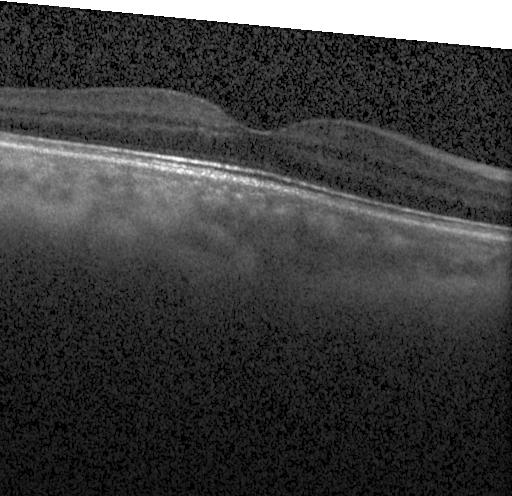
Spectral-domain optical coherence tomography; optical coherence tomography B-scan; through the macula; Heidelberg Spectralis OCT system.
Assessment: neither choroidal neovascularization, diabetic macular edema, nor drusen.